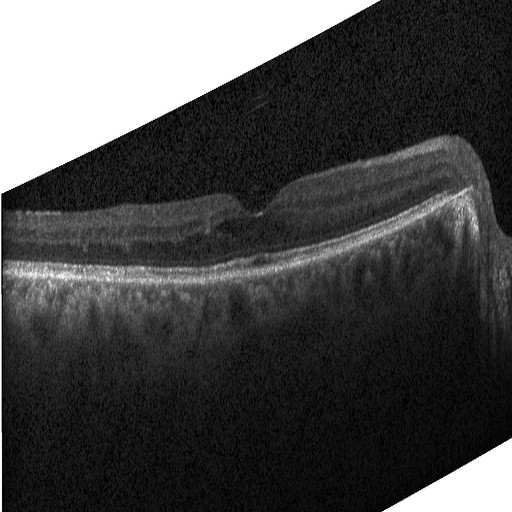 Fovea-centered. OCT B-scan. SD-OCT. Acquired on a Heidelberg Spectralis.
Macular OCT: diabetic macular edema.